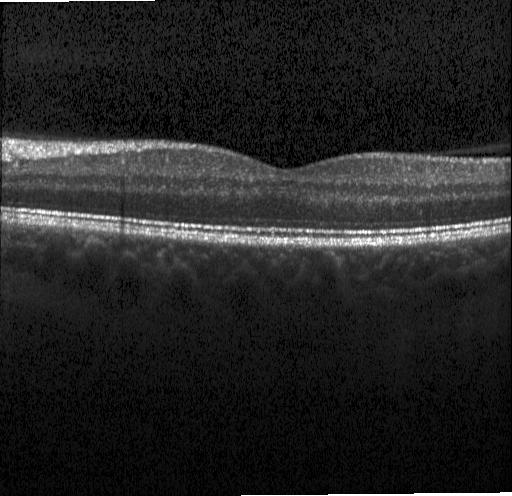 SD-OCT; OCT B-scan
Assessment: no CNV, DME, or drusen.